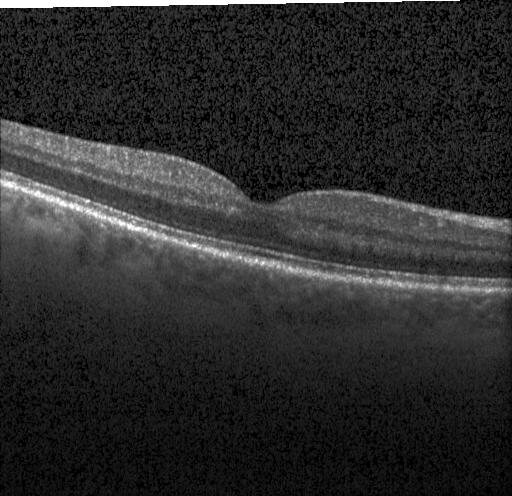 Spectral-domain OCT B-scan: no choroidal neovascularization, diabetic macular edema, or drusen.